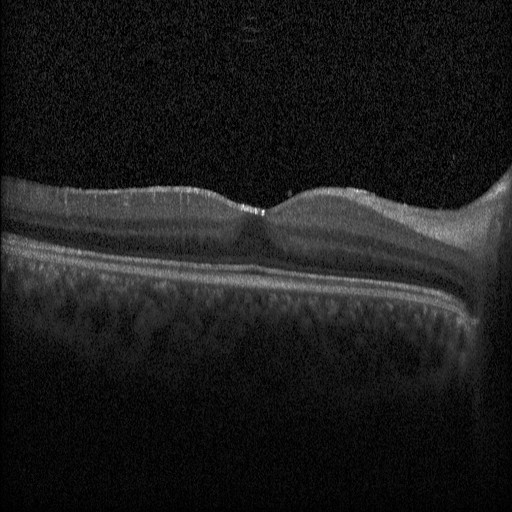 Instrument: Heidelberg Spectralis, retinal OCT cross-section, spectral-domain optical coherence tomography, fovea-centered. Diagnosis: DME.